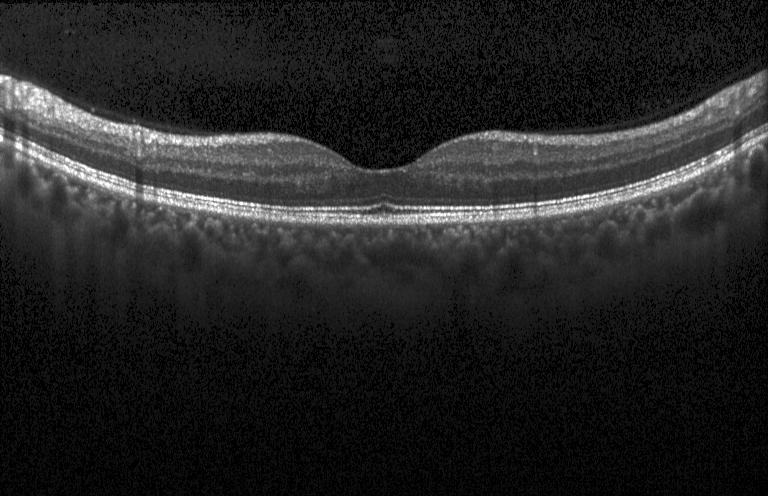 Diagnosis: no choroidal neovascularization, no diabetic macular edema, and no drusen.